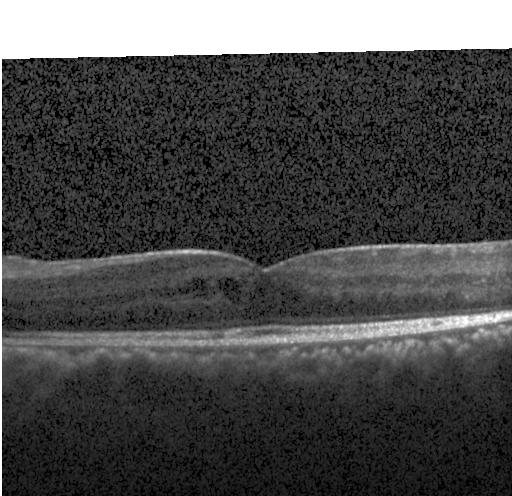
Spectral-domain OCT B-scan: diabetic macular edema.